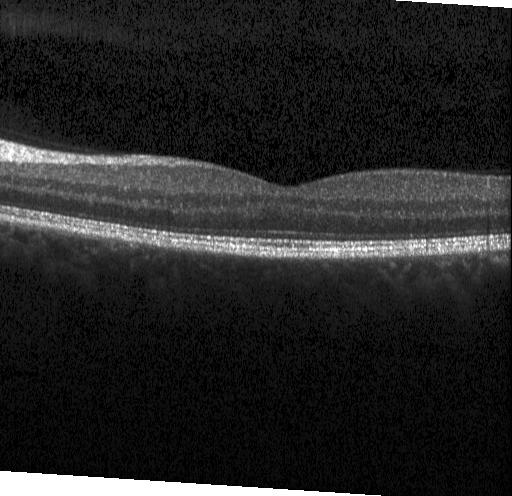

Retinal OCT B-scan; Heidelberg Spectralis OCT system; spectral-domain OCT; through the macula — No evidence of choroidal neovascularization, diabetic macular edema, or drusen.